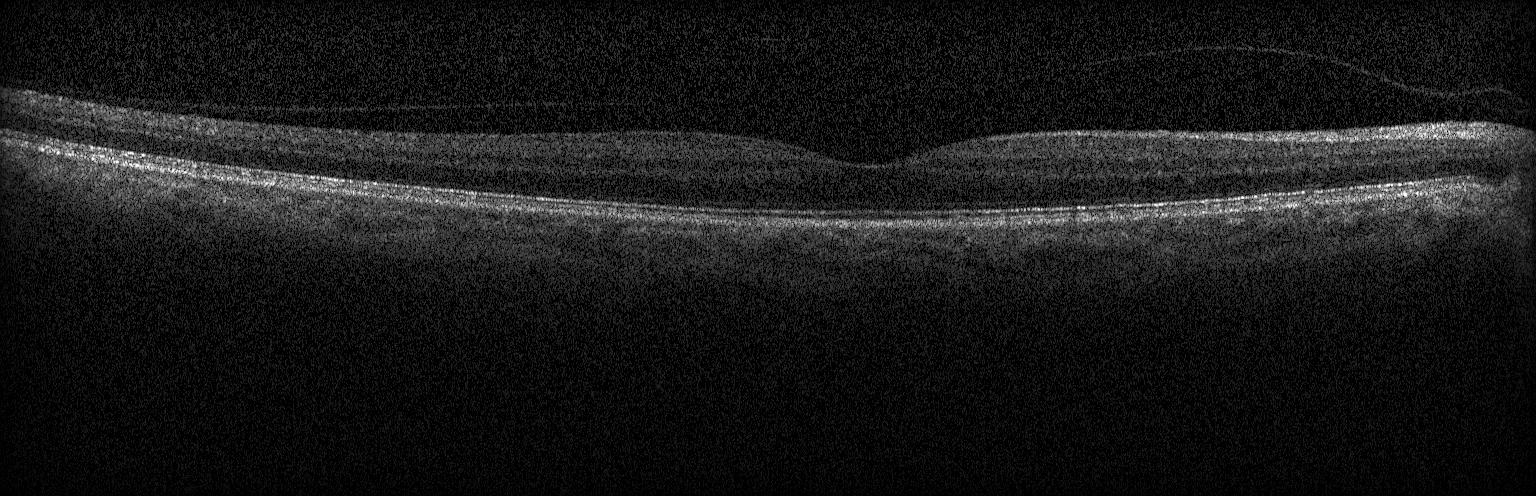 Retinal OCT B-scan; instrument: Heidelberg Spectralis — Assessment: no evidence of choroidal neovascularization, diabetic macular edema, or drusen.